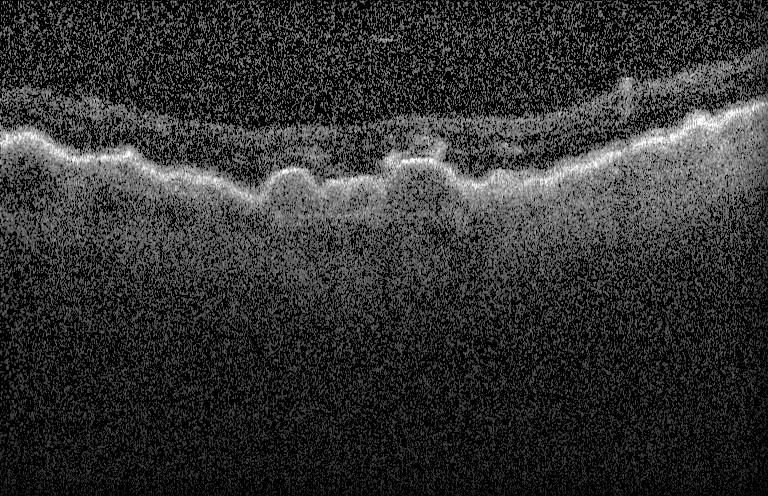
Finding: a choroidal neovascular membrane.